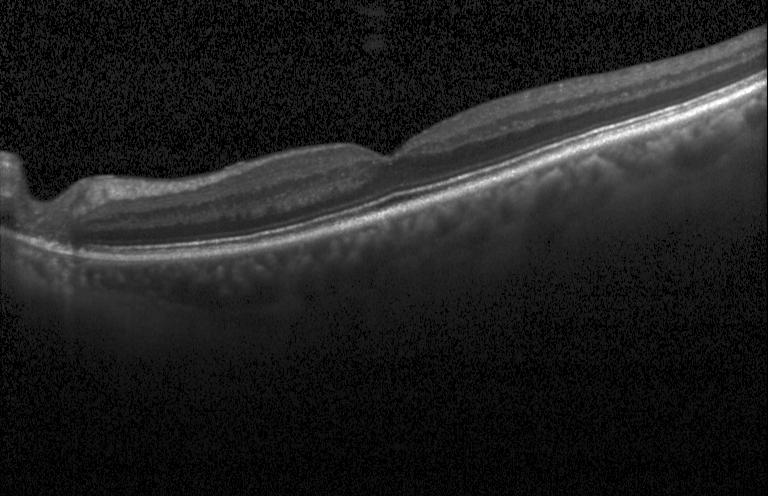
Retinal OCT cross-section. Finding: no choroidal neovascularization, no diabetic macular edema, and no drusen.